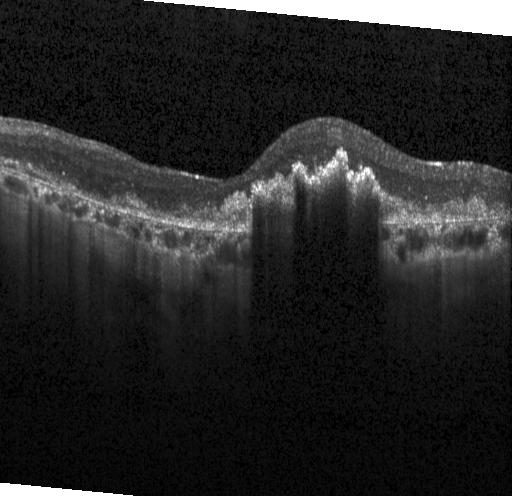
Impression: a choroidal neovascular membrane.